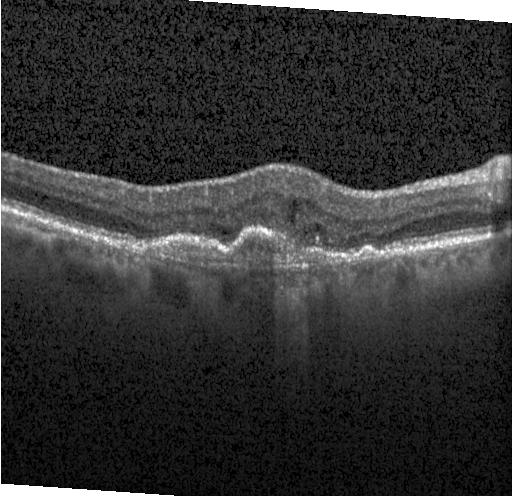 Optical coherence tomography scan. SD-OCT
Diagnosis: a choroidal neovascular membrane.